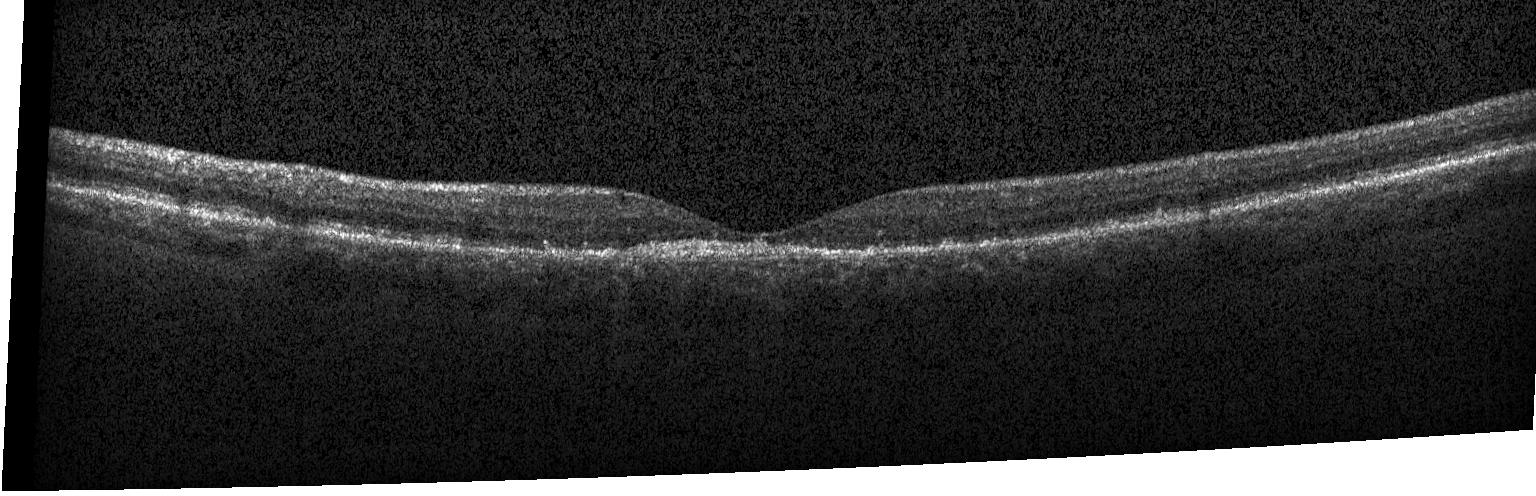

Through the macula; SD-OCT; acquired on a Heidelberg Spectralis; retinal OCT cross-section.
Impression: CNV.